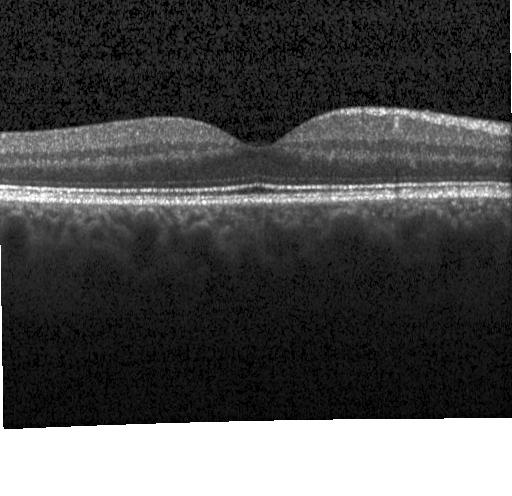
This B-scan demonstrates no evidence of choroidal neovascularization, diabetic macular edema, or drusen.